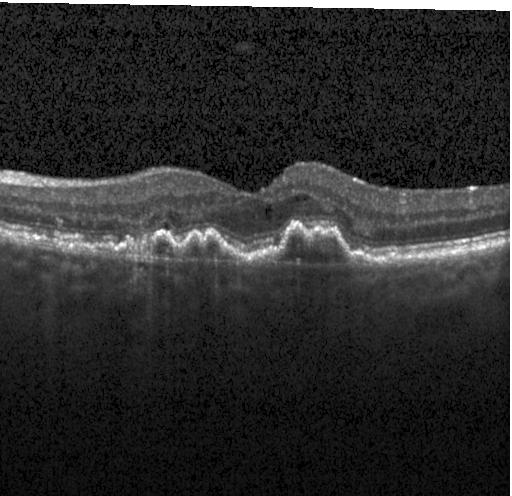
Dx: choroidal neovascularization (CNV).